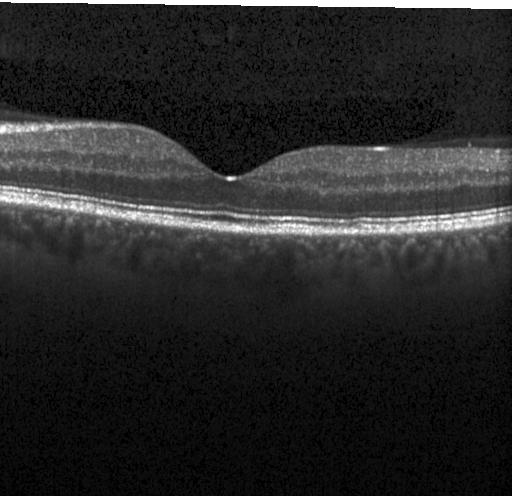
OCT finding: no choroidal neovascularization, no diabetic macular edema, and no drusen.